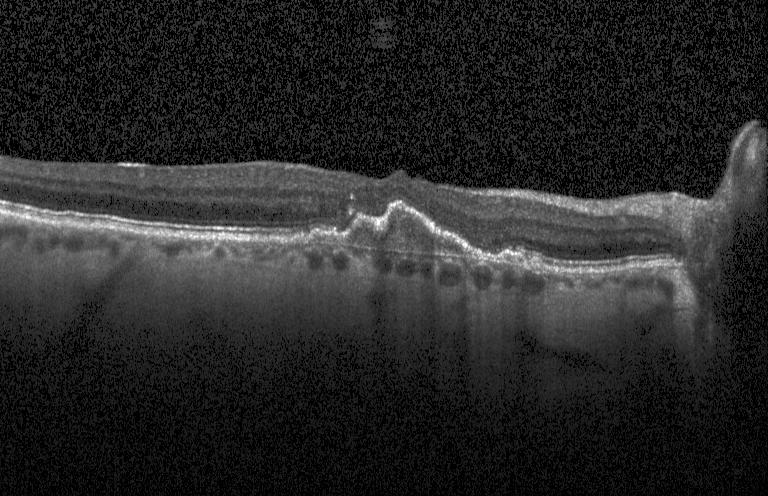
Macular OCT: a choroidal neovascular membrane.